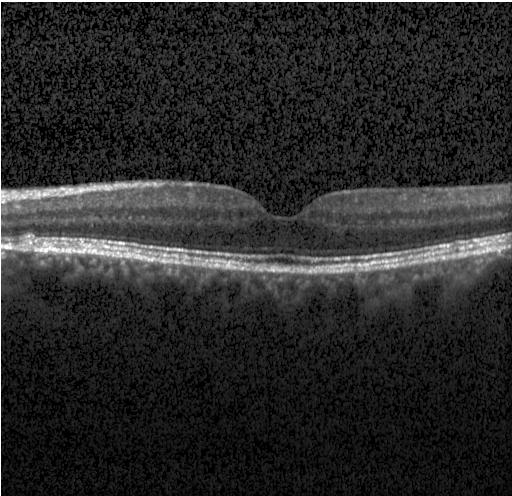
Optical coherence tomography B-scan. SD-OCT. Centered on the fovea
Impression: no choroidal neovascularization, no diabetic macular edema, and no drusen.